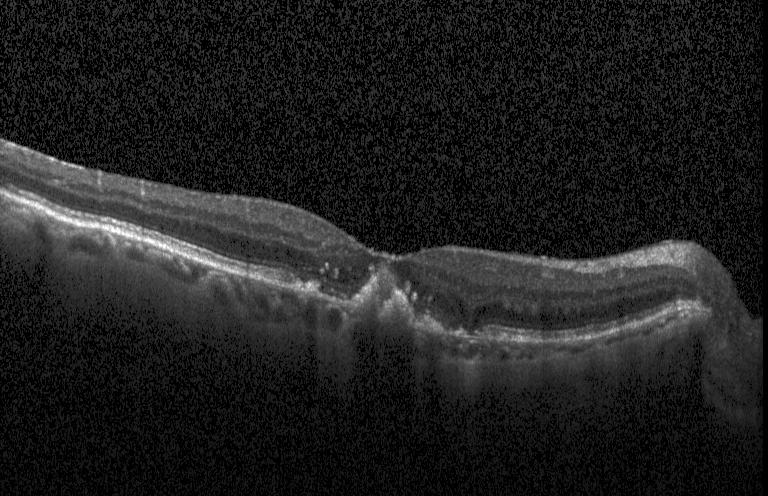
Horizontal scan through the fovea. OCT B-scan — Dx: choroidal neovascularization.